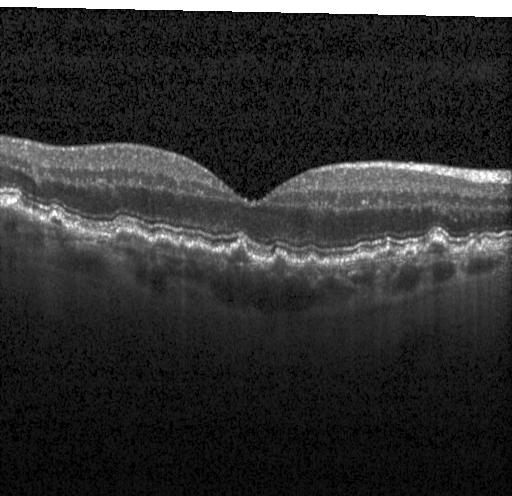

Retinal OCT cross-section. Diagnosis: drusen.